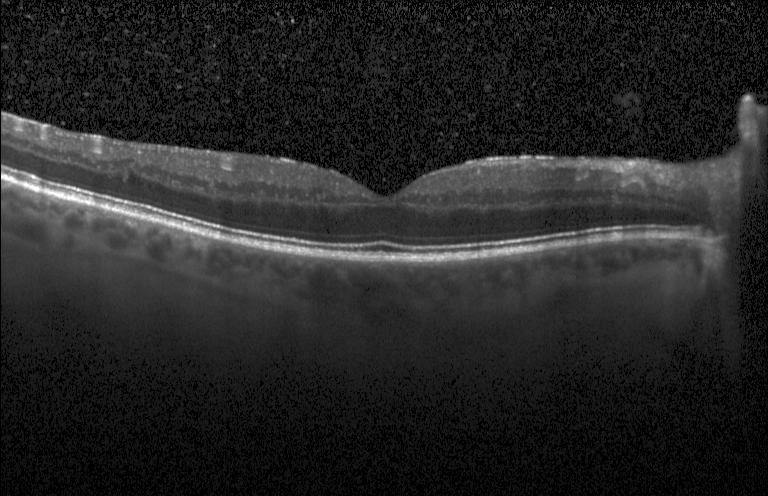

OCT finding: no evidence of choroidal neovascularization, diabetic macular edema, or drusen.